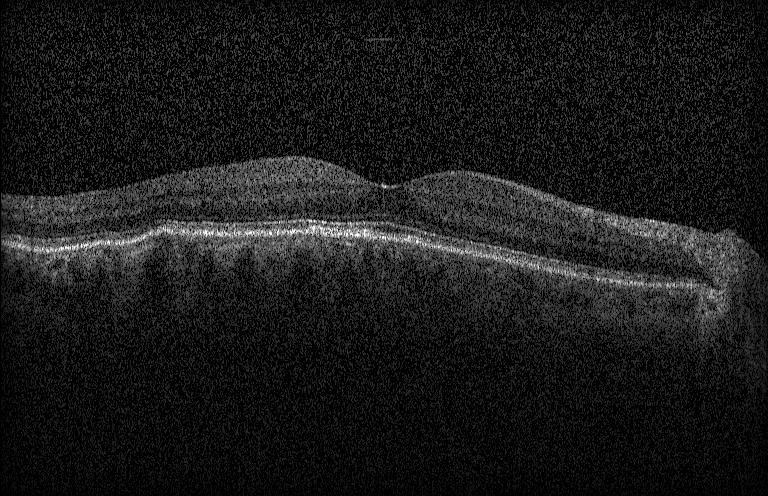
Spectral-domain optical coherence tomography · Heidelberg Spectralis · horizontal scan through the fovea · OCT B-scan
This B-scan demonstrates no choroidal neovascularization, diabetic macular edema, or drusen.